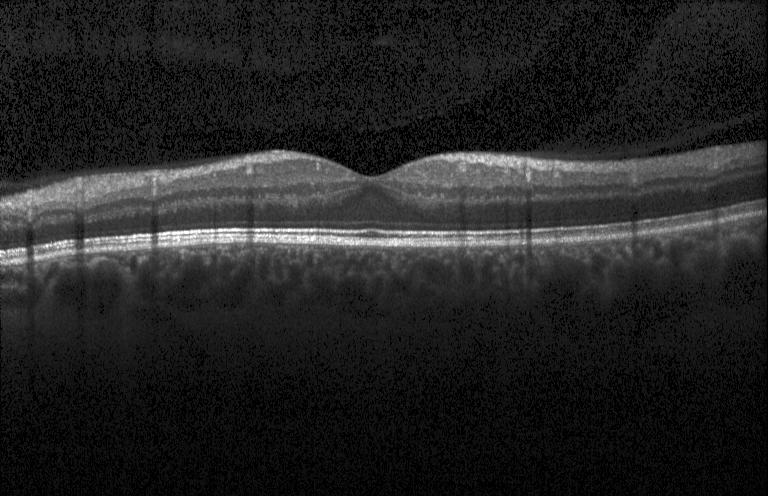 Optical coherence tomography scan
Diagnosis: neither CNV, DME, nor drusen.